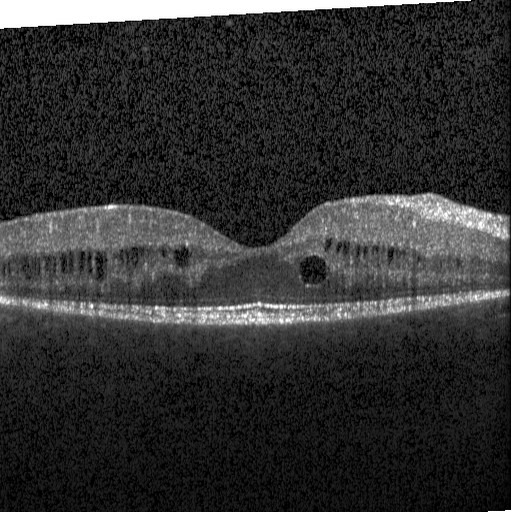
Retinal OCT B-scan.
Diabetic macular edema (DME).